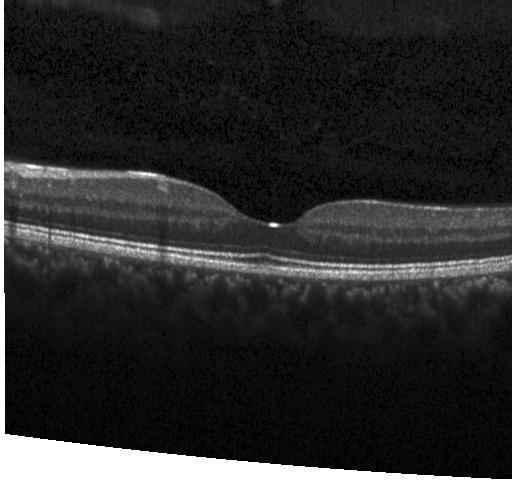

Impression: no evidence of CNV, DME, or drusen.